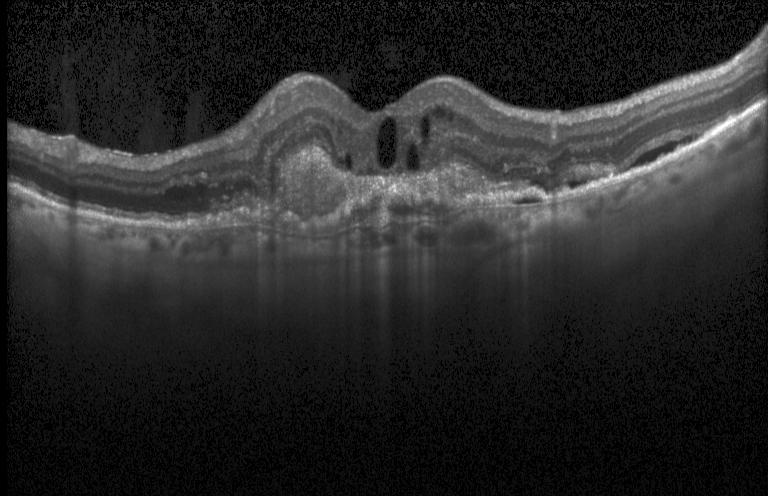 Finding: choroidal neovascularization (CNV).